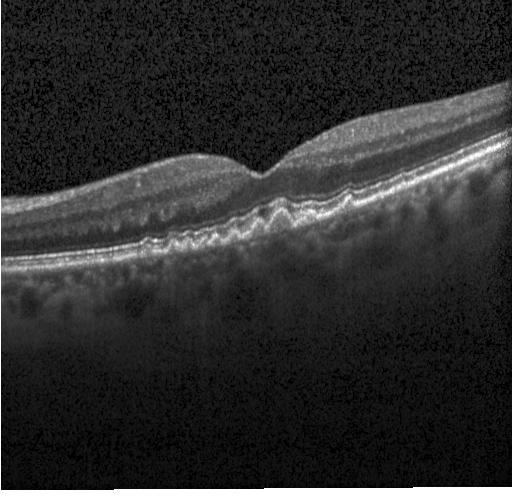
Retinal OCT cross-section; Heidelberg Spectralis OCT system; through the macula; spectral-domain OCT — Dx: drusen.